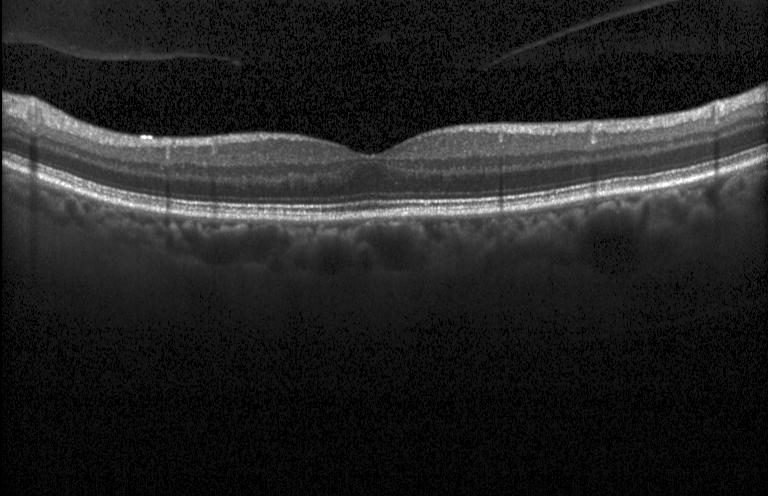

Through the macula. Acquired on a Heidelberg Spectralis. SD-OCT. Retinal OCT B-scan. No choroidal neovascularization, diabetic macular edema, or drusen.